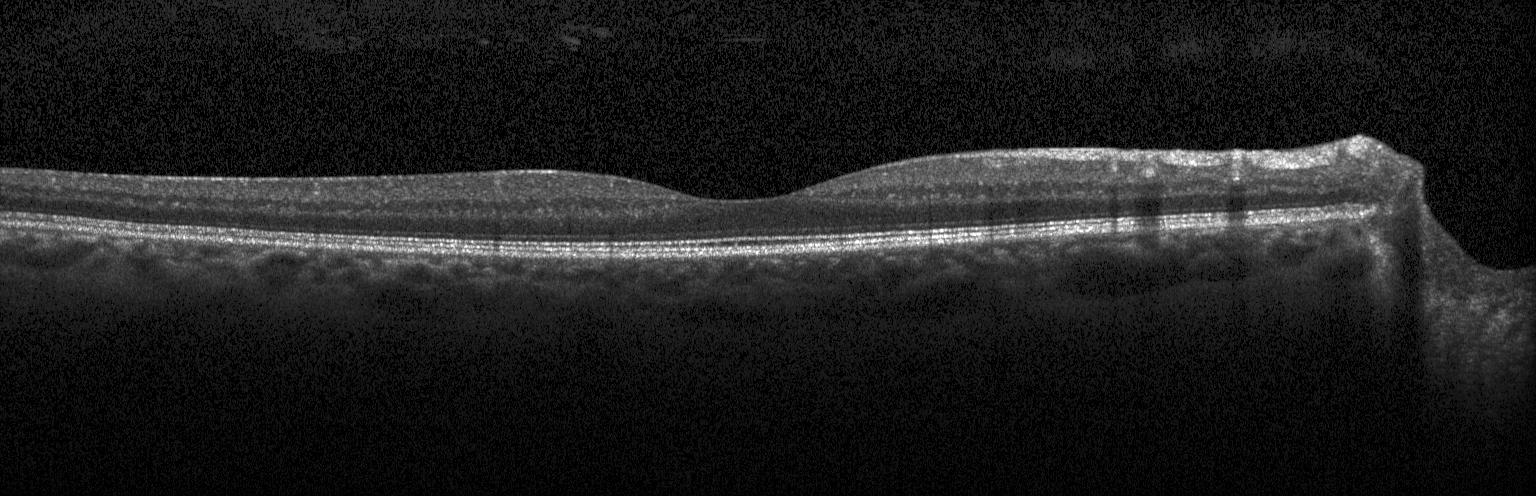

Retinal OCT B-scan — Diagnosis: no evidence of choroidal neovascularization, diabetic macular edema, or drusen.